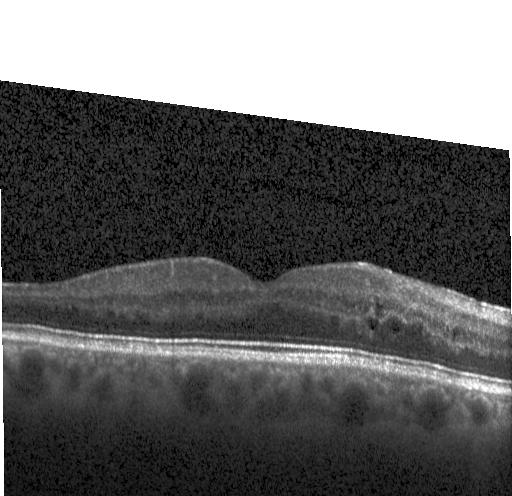
Horizontal scan through the fovea, retinal OCT cross-section, SD-OCT.
Dx: DME.